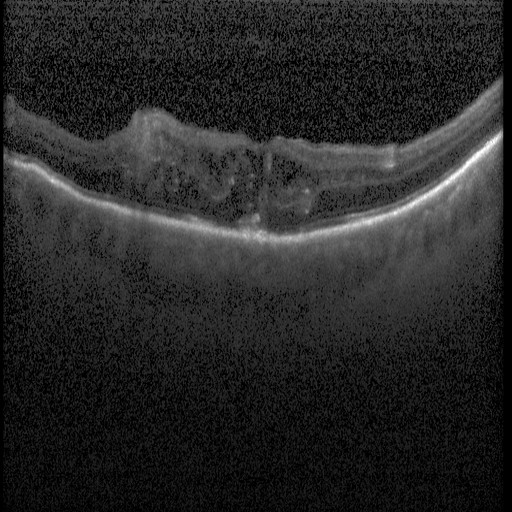

Through the macula; retinal OCT B-scan; SD-OCT. Diabetic macular edema (DME).